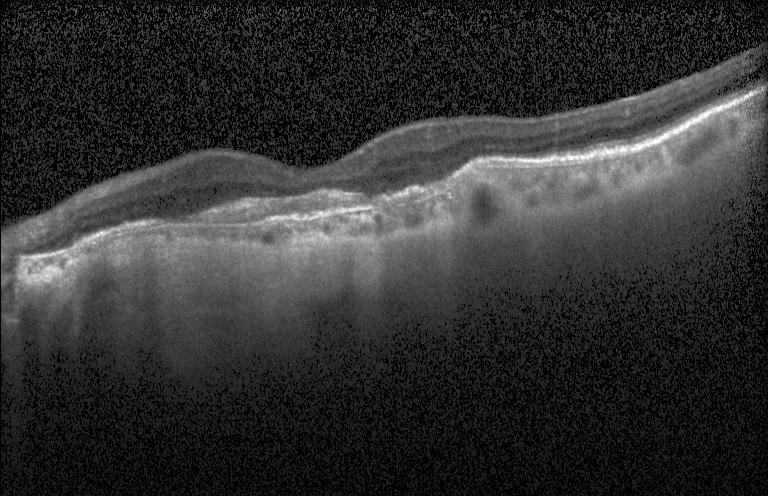
The scan shows choroidal neovascularization.